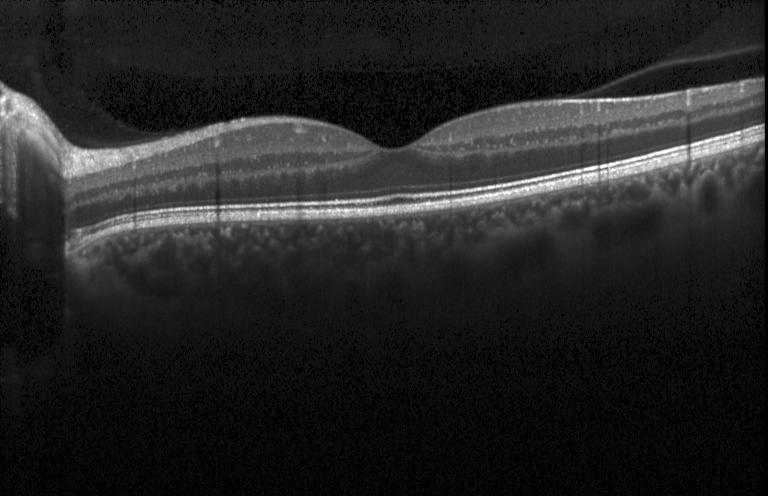 Acquired on a Heidelberg Spectralis · OCT line scan · spectral-domain optical coherence tomography
Impression: no CNV, no DME, and no drusen.